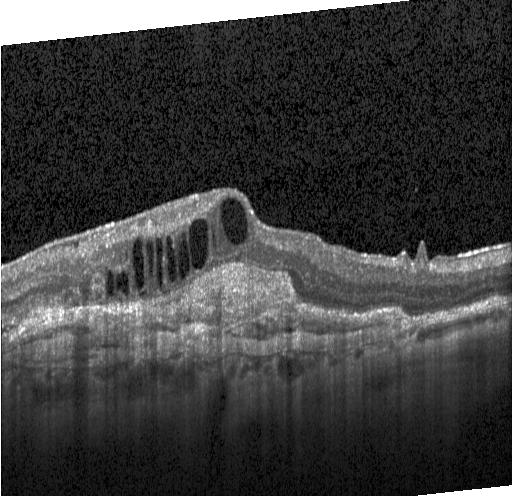

Spectral-domain OCT; instrument: Heidelberg Spectralis; horizontal scan through the fovea; optical coherence tomography B-scan.
Finding: CNV.